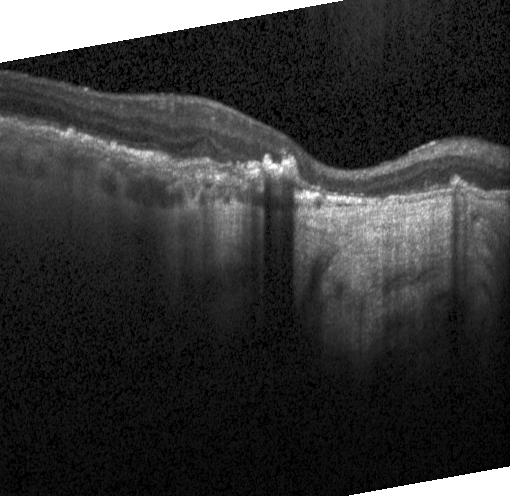

Retinal OCT B-scan. Diagnosis: CNV.